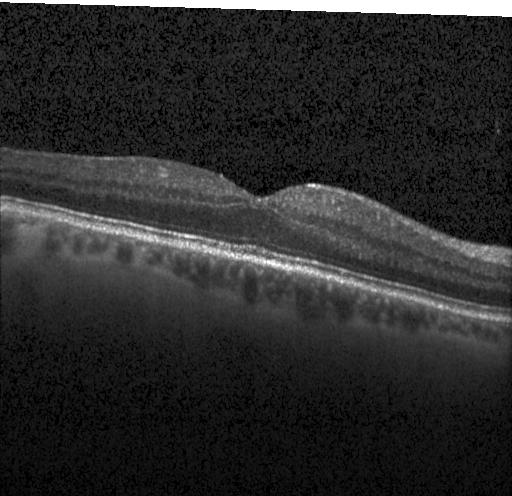
Macular scan; Heidelberg Spectralis; optical coherence tomography scan.
Diagnosis: no choroidal neovascularization, diabetic macular edema, or drusen.